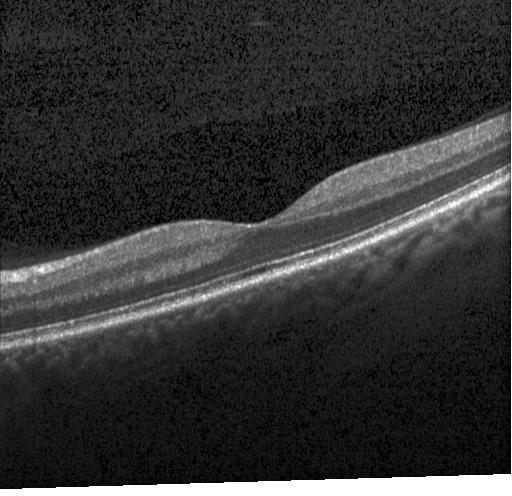

Retinal OCT B-scan.
Diagnosis: no choroidal neovascularization, no diabetic macular edema, and no drusen.